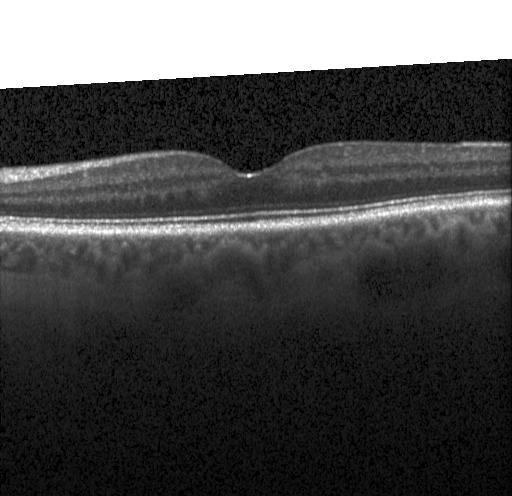
OCT finding: no choroidal neovascularization, no diabetic macular edema, and no drusen.